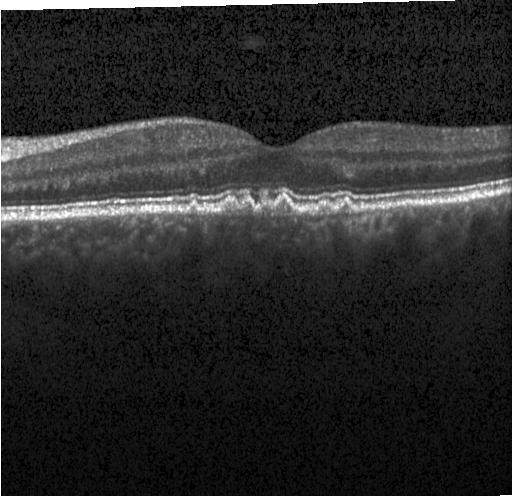 Spectral-domain optical coherence tomography, acquired on a Heidelberg Spectralis, OCT line scan. Multiple drusen.